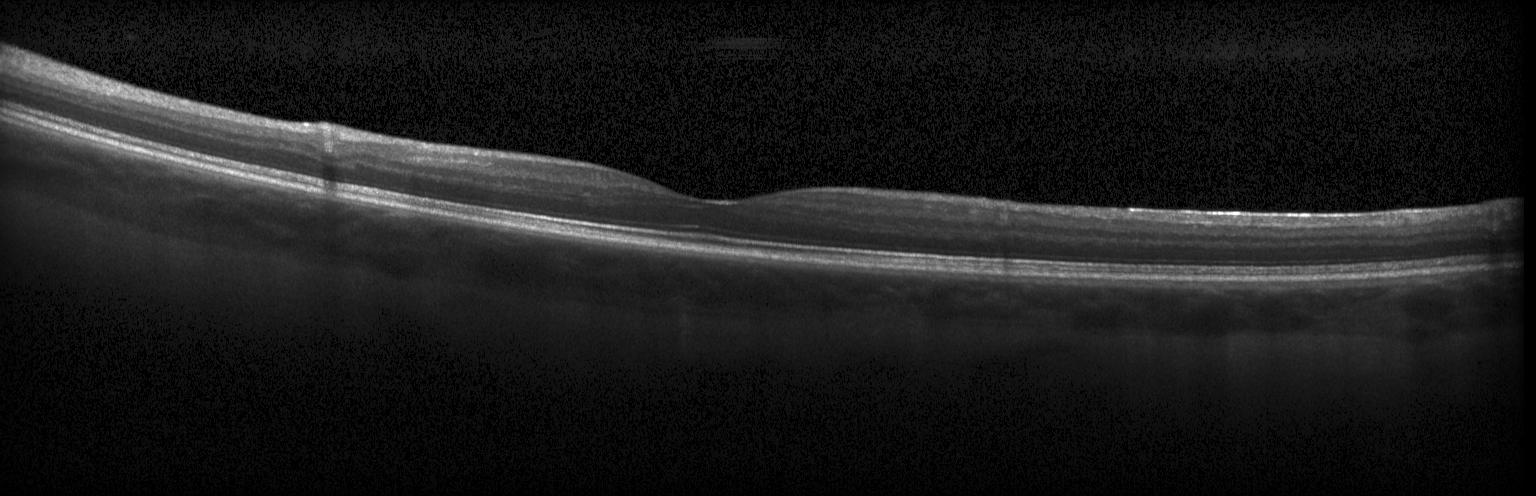 OCT B-scan. Impression: neither choroidal neovascularization, diabetic macular edema, nor drusen.